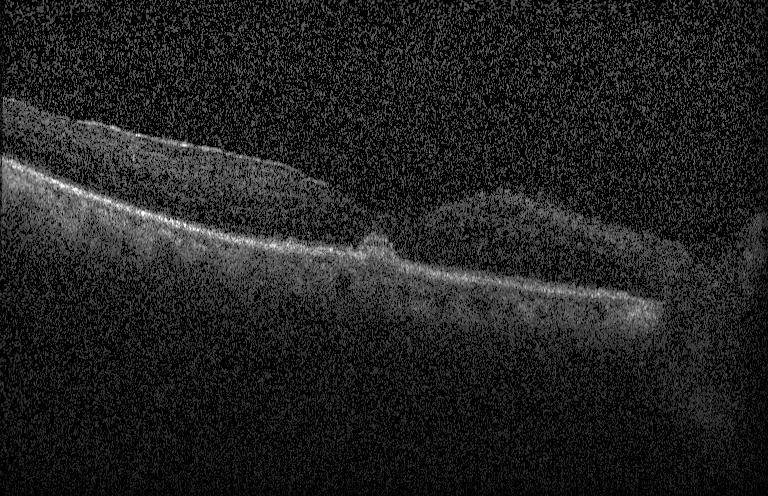

Optical coherence tomography B-scan — OCT finding: a choroidal neovascular membrane.